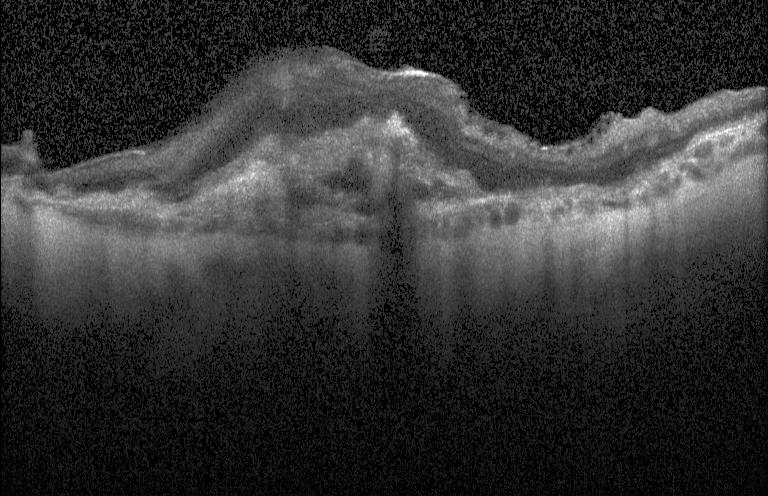
OCT line scan.
The scan shows a choroidal neovascular membrane.